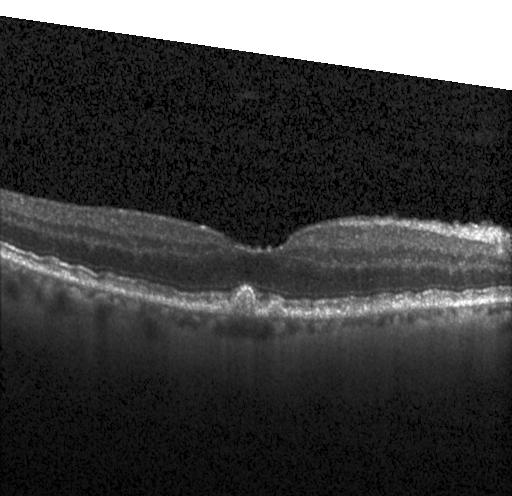
The scan shows drusen.